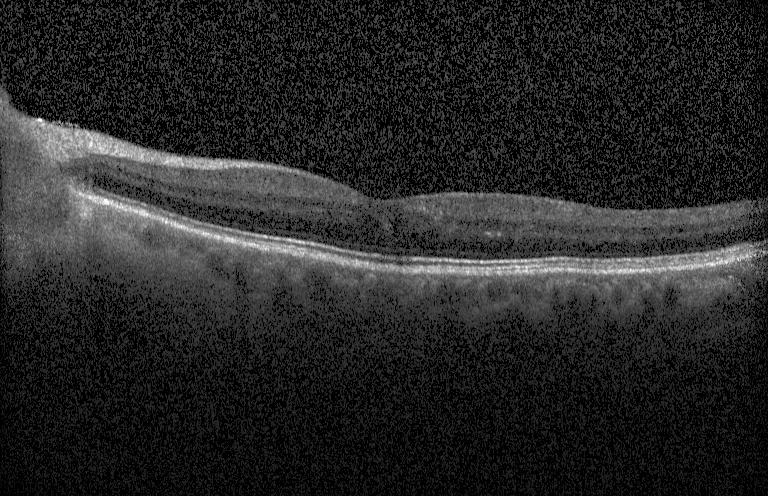
SD-OCT, OCT line scan.
Assessment: no evidence of choroidal neovascularization, diabetic macular edema, or drusen.